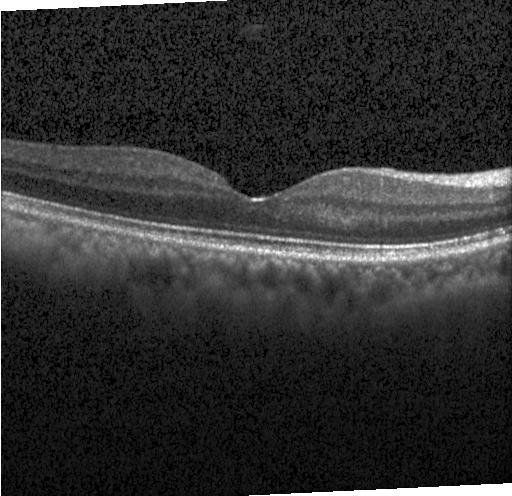 Impression: no evidence of choroidal neovascularization, diabetic macular edema, or drusen.